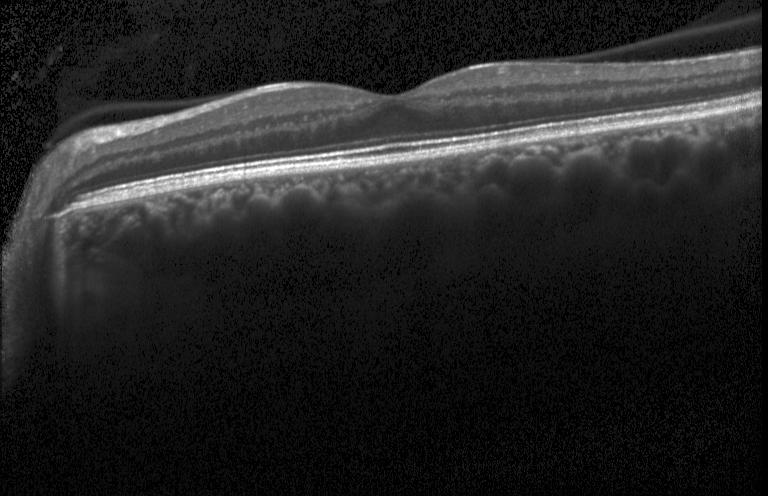 Optical coherence tomography scan — Neither CNV, DME, nor drusen.